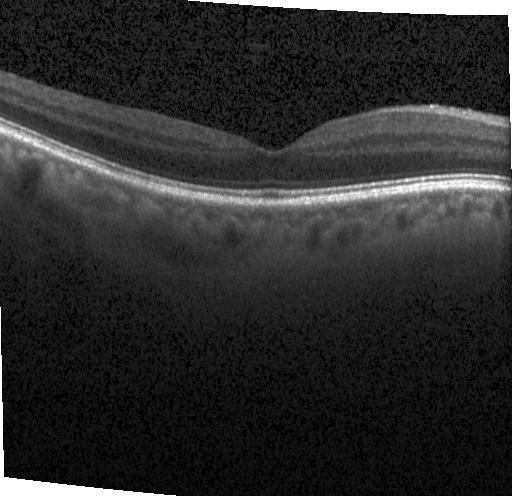 Spectral-domain OCT · retinal OCT cross-section · through the macula.
Finding: no choroidal neovascularization, diabetic macular edema, or drusen.